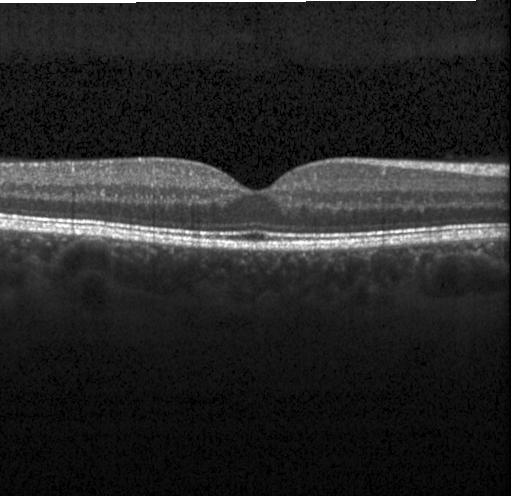 Optical coherence tomography scan
Impression: no choroidal neovascularization, diabetic macular edema, or drusen.